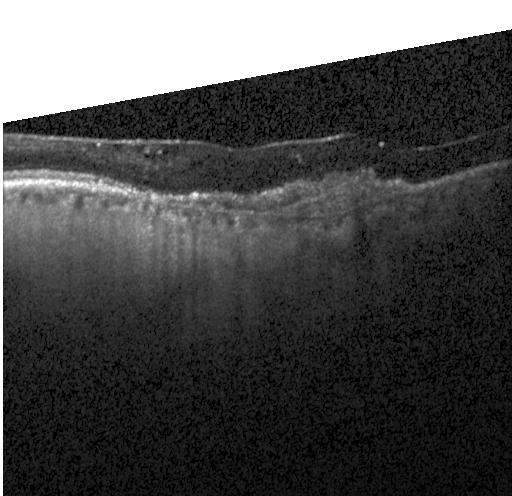 The scan shows choroidal neovascularization (CNV).